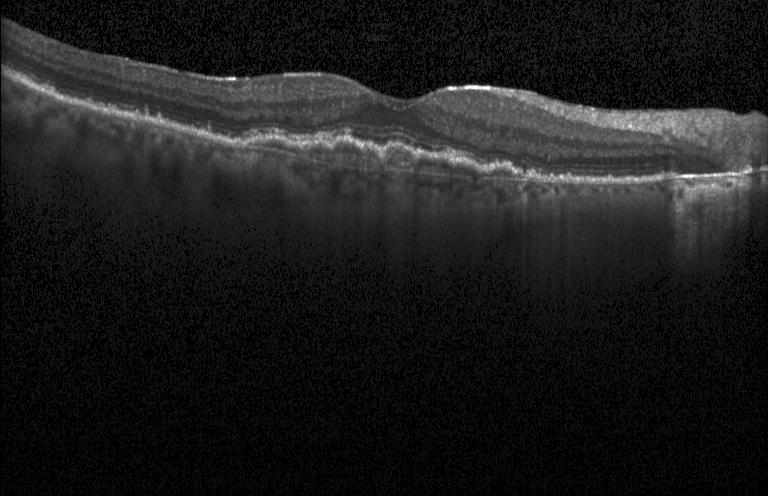
Instrument: Heidelberg Spectralis · retinal OCT B-scan · macular scan.
Assessment: choroidal neovascularization.